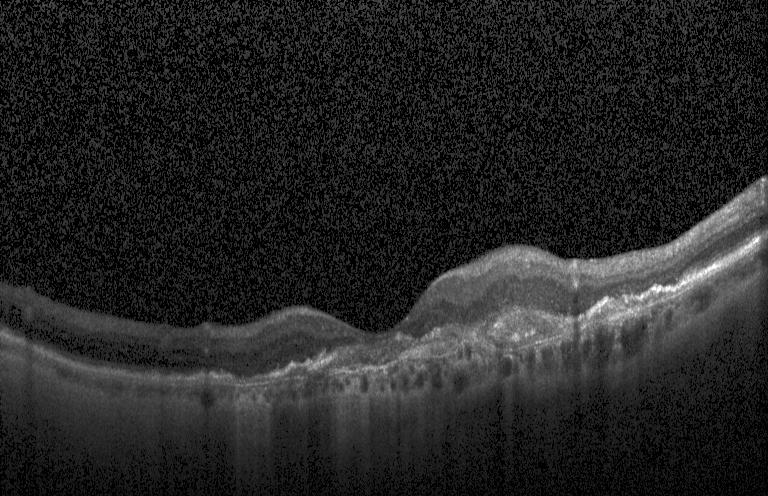 Macular OCT: choroidal neovascularization.